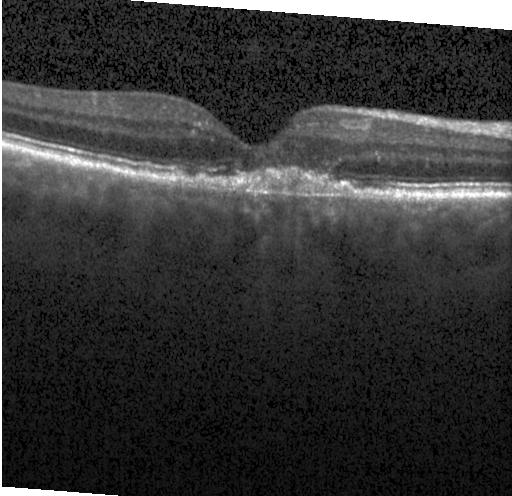
Retinal OCT cross-section, macular scan.
Finding: a choroidal neovascular membrane.